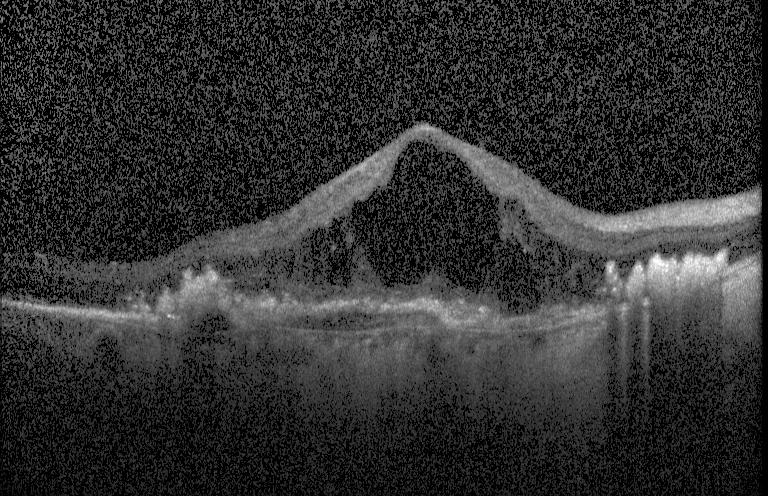 OCT line scan; Heidelberg Spectralis; spectral-domain OCT; fovea-centered. Impression: choroidal neovascularization.